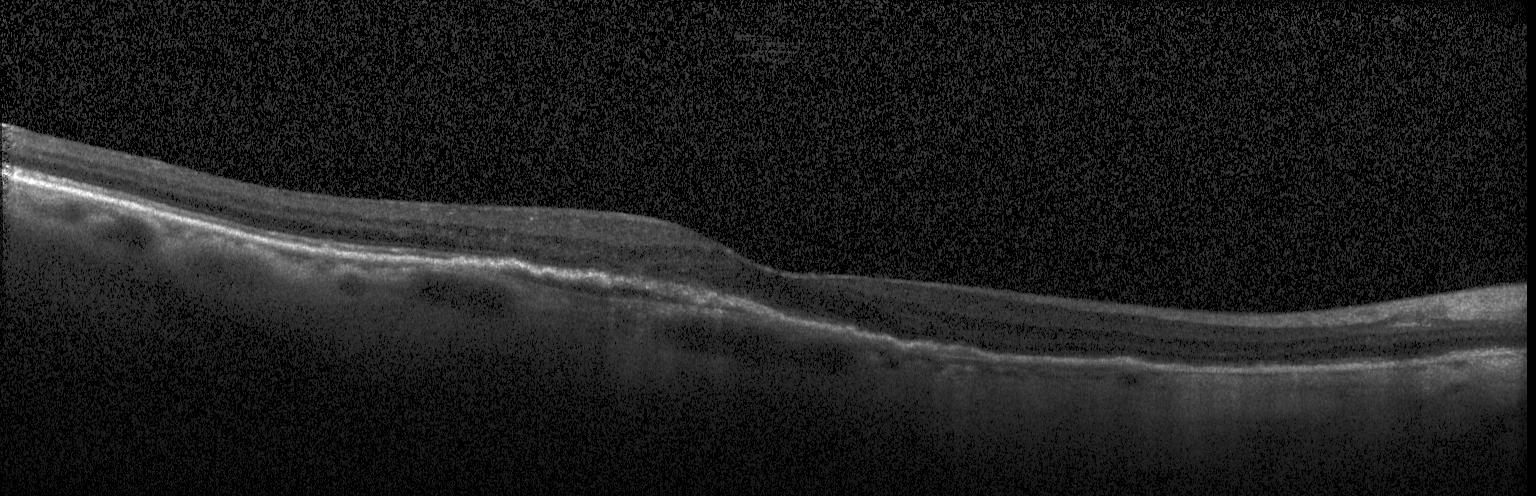

Optical coherence tomography scan; instrument: Heidelberg Spectralis; spectral-domain optical coherence tomography.
Impression: choroidal neovascularization.